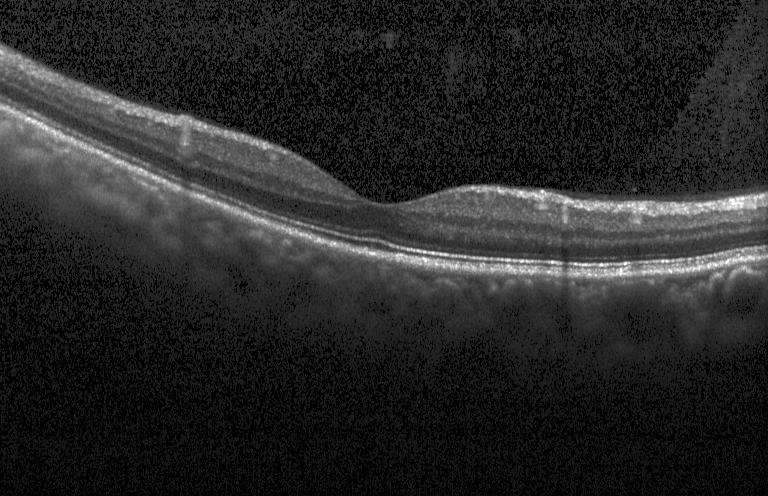

OCT B-scan
OCT finding: no evidence of choroidal neovascularization, diabetic macular edema, or drusen.